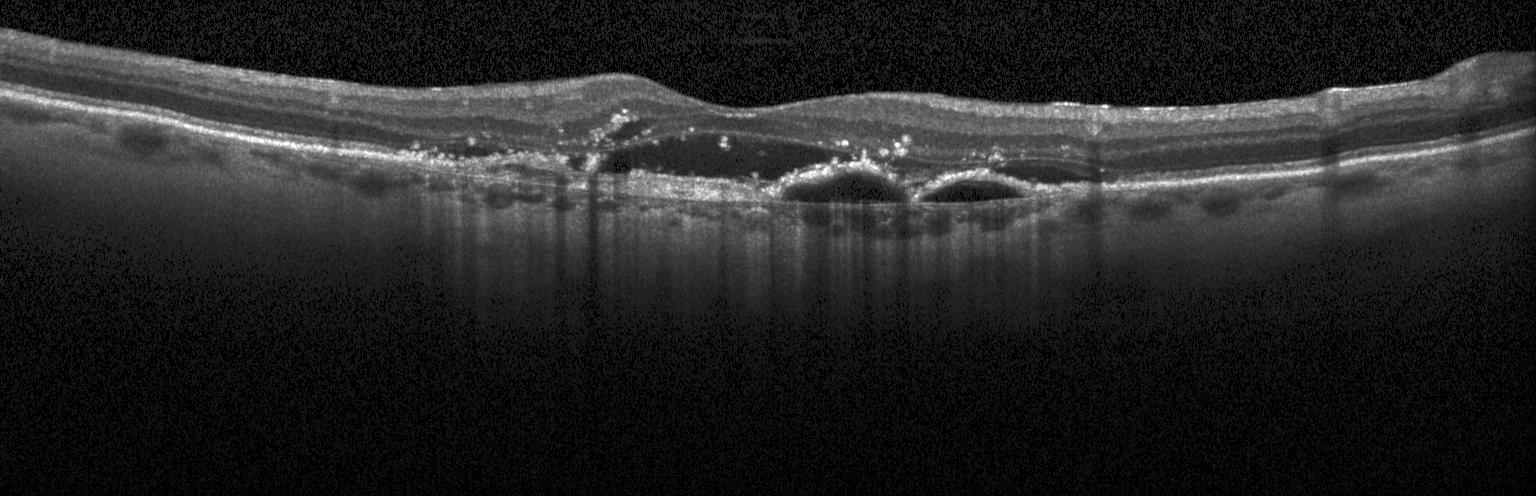

Diagnosis: CNV.